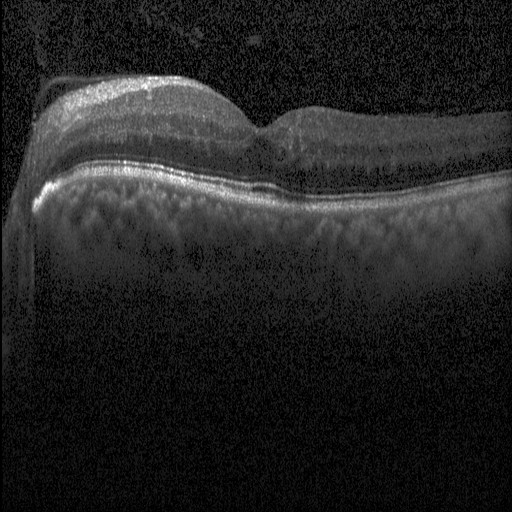 Retinal OCT cross-section — Diabetic macular edema (DME).